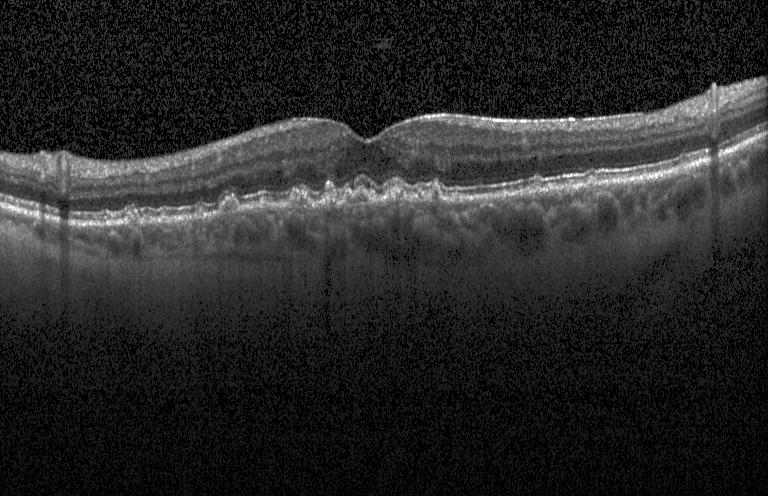

Optical coherence tomography B-scan · SD-OCT. Impression: multiple drusen.